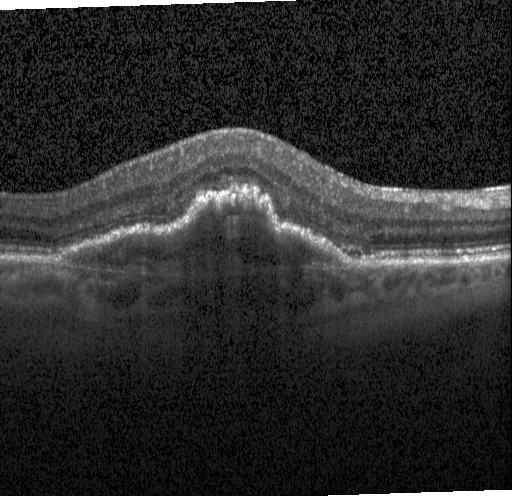

OCT finding: a choroidal neovascular membrane.